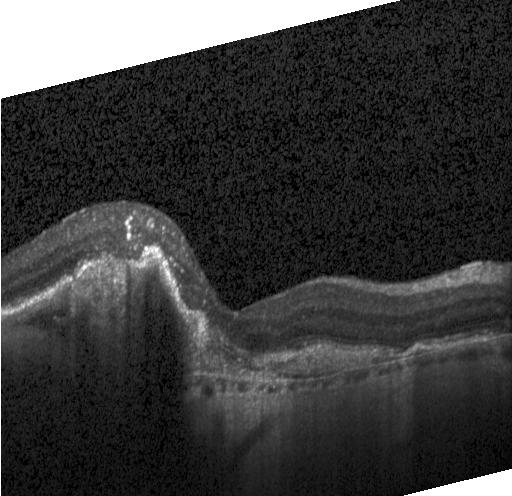

Heidelberg Spectralis · retinal OCT cross-section · spectral-domain OCT · through the macula. This B-scan demonstrates a choroidal neovascular membrane.